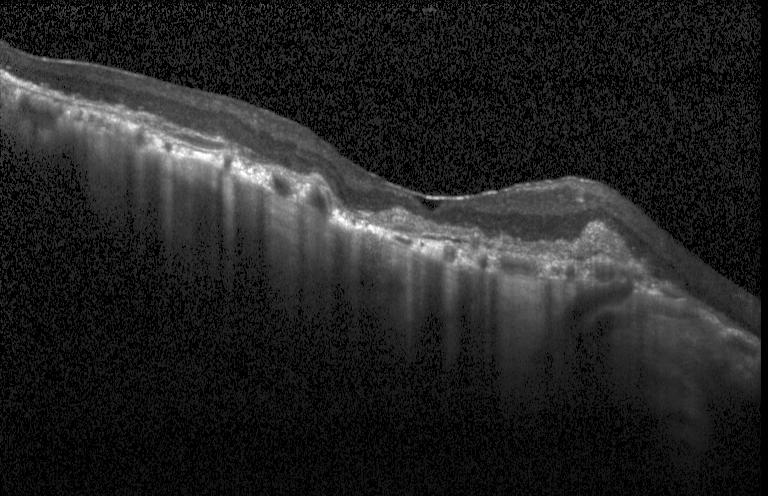

OCT line scan, SD-OCT, Heidelberg Spectralis OCT system
This B-scan demonstrates choroidal neovascularization.